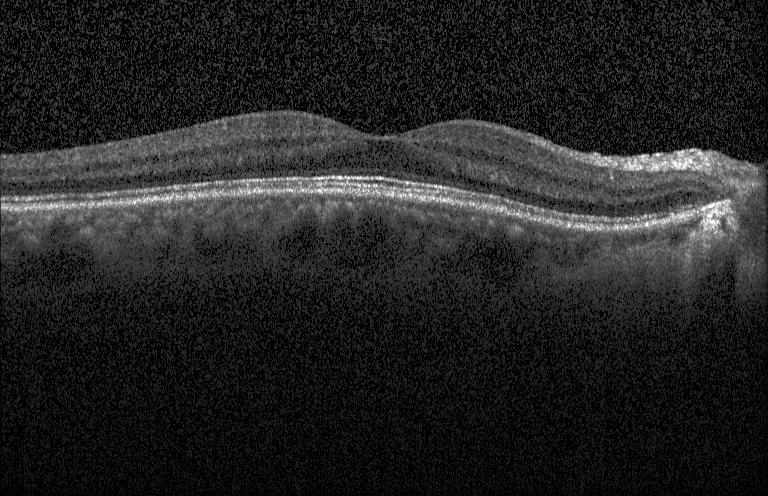
Retinal OCT cross-section.
Assessment: no CNV, no DME, and no drusen.